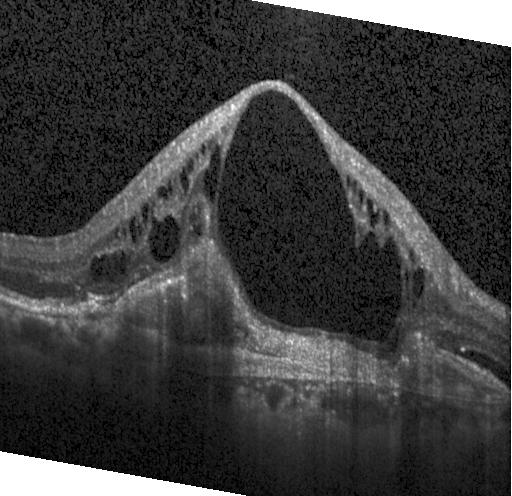 Retinal OCT B-scan. Centered on the fovea — Macular OCT: a choroidal neovascular membrane.